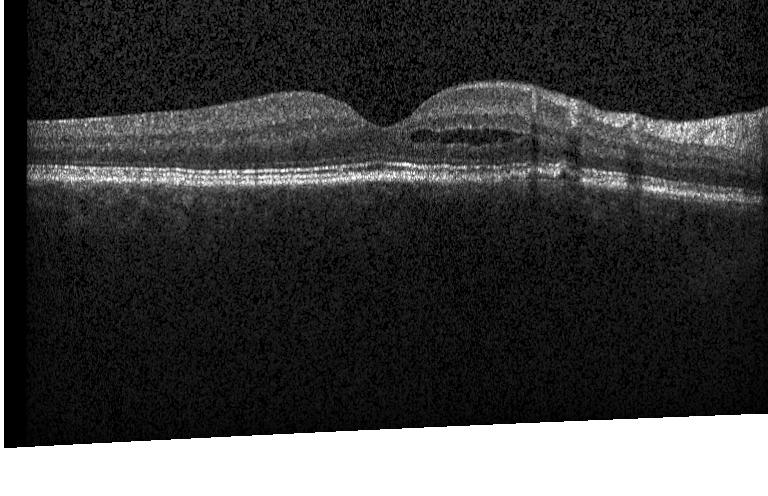
Retinal OCT cross-section · spectral-domain optical coherence tomography · instrument: Heidelberg Spectralis · fovea-centered — Finding: a choroidal neovascular membrane.